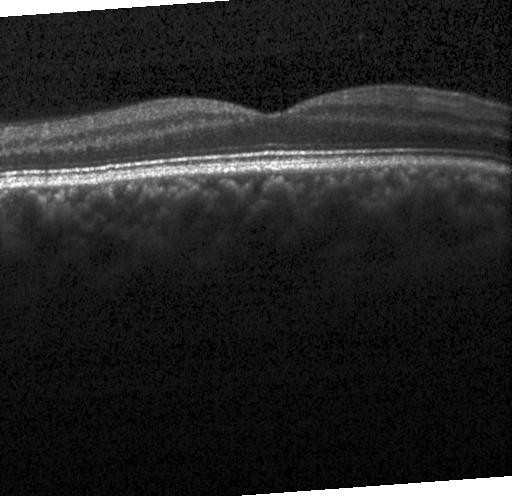

OCT line scan; SD-OCT. Assessment: no choroidal neovascularization, no diabetic macular edema, and no drusen.